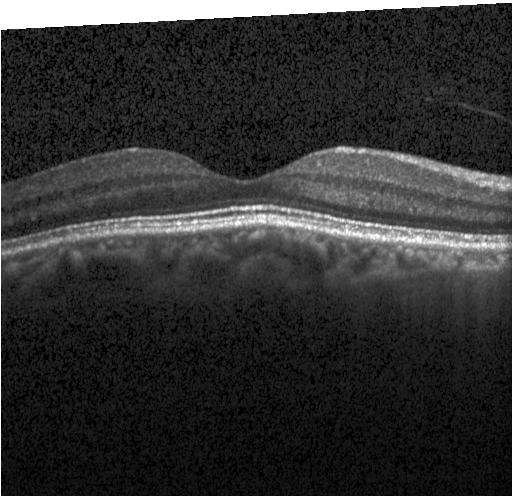

Diagnosis: no evidence of choroidal neovascularization, diabetic macular edema, or drusen.